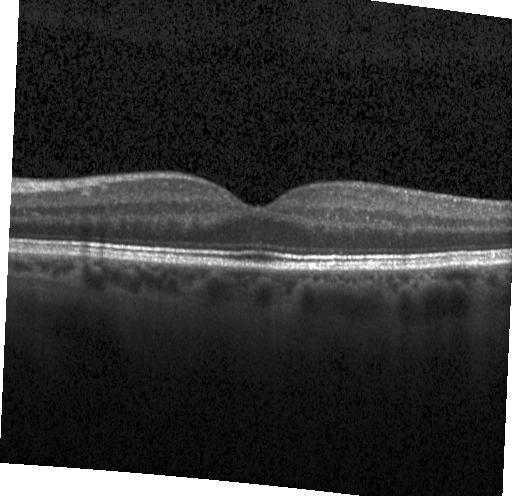

Spectral-domain OCT; Heidelberg Spectralis OCT system; macular scan; optical coherence tomography scan.
Dx: no CNV, no DME, and no drusen.